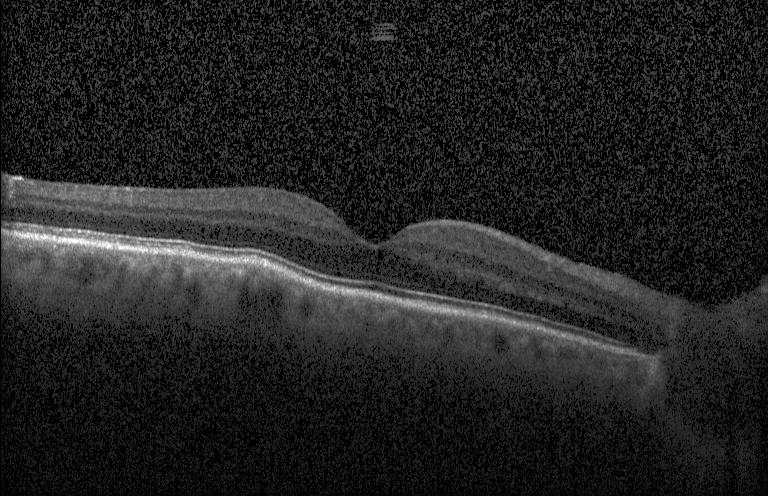

Finding: no evidence of choroidal neovascularization, diabetic macular edema, or drusen.